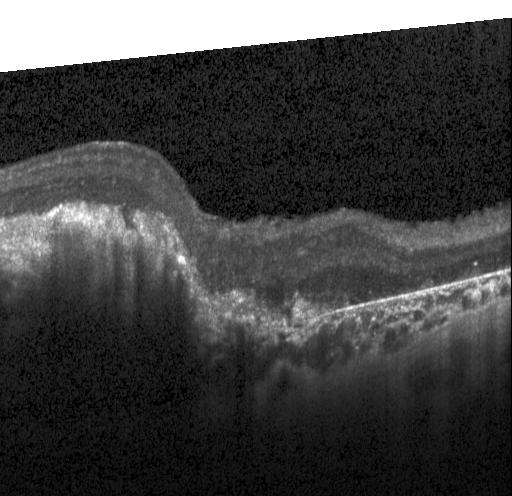 Spectral-domain optical coherence tomography; optical coherence tomography scan; fovea-centered
Assessment: a choroidal neovascular membrane.